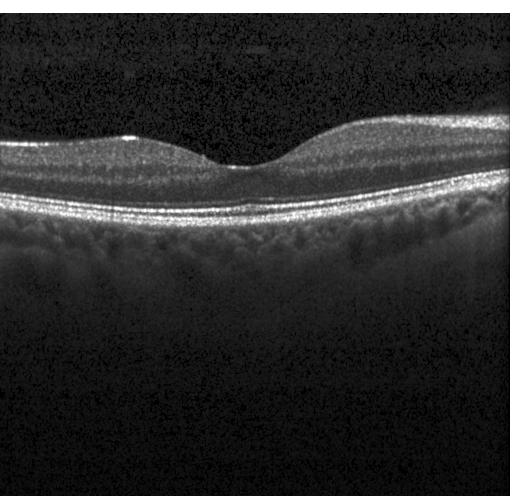

Finding: neither choroidal neovascularization, diabetic macular edema, nor drusen.